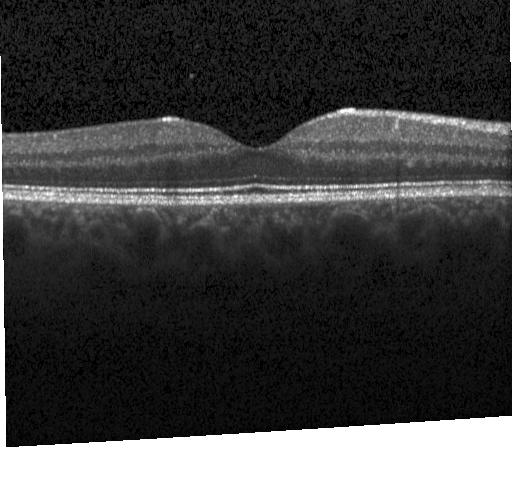 Macular OCT: neither choroidal neovascularization, diabetic macular edema, nor drusen.